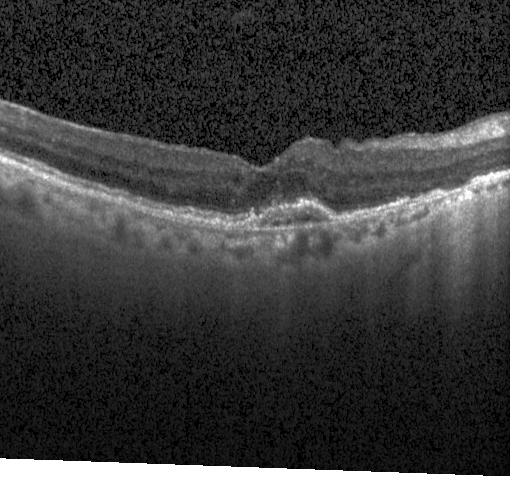 Spectral-domain OCT · OCT line scan · Heidelberg Spectralis · fovea-centered. This B-scan demonstrates CNV.